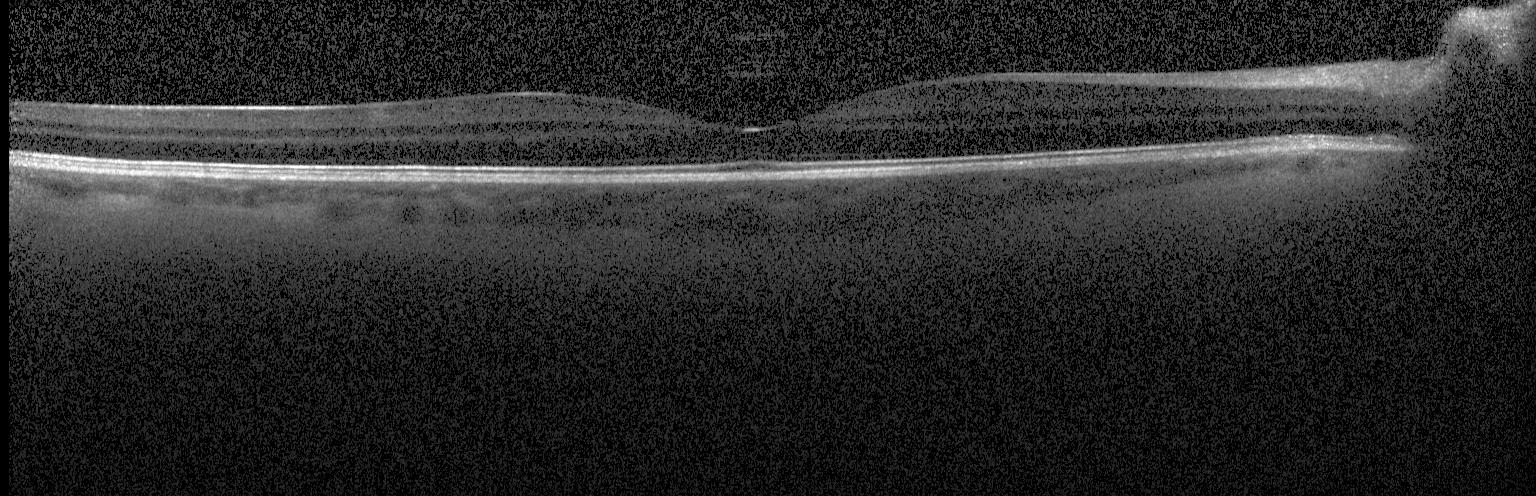

OCT B-scan showing neither choroidal neovascularization, diabetic macular edema, nor drusen.